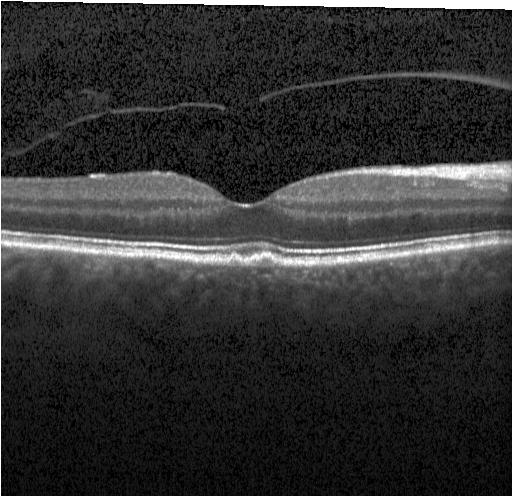 This B-scan demonstrates sub-RPE drusenoid deposits.